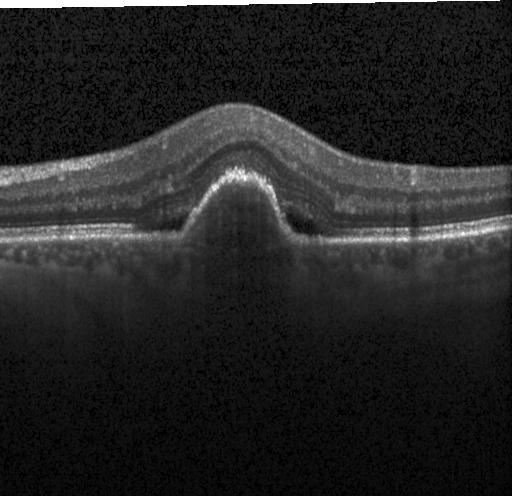
Retinal OCT cross-section showing choroidal neovascularization.